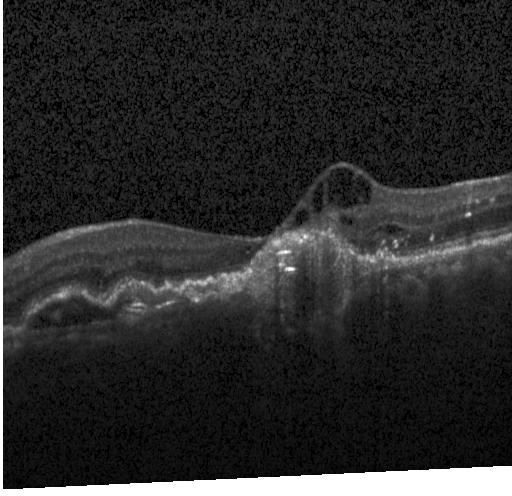 SD-OCT · OCT B-scan · horizontal scan through the fovea
OCT finding: choroidal neovascularization.